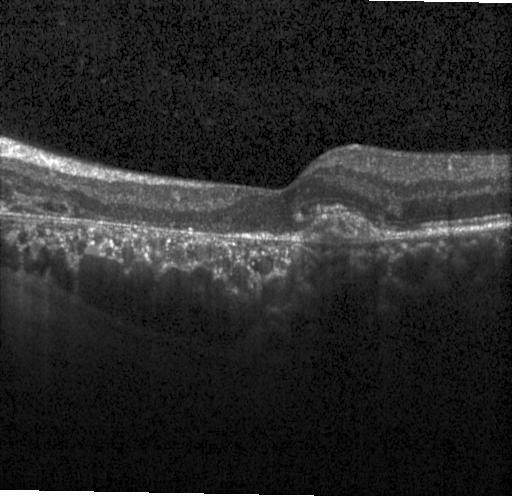

Diagnosis: choroidal neovascularization.